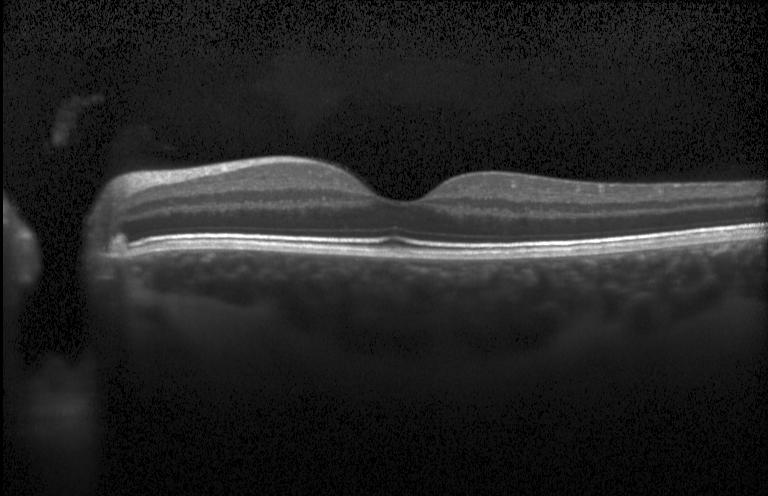 OCT finding: no evidence of CNV, DME, or drusen.